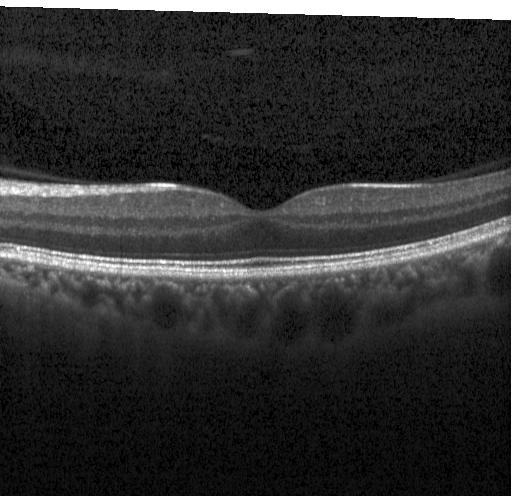

Macular scan. OCT B-scan. Heidelberg Spectralis. SD-OCT
Diagnosis: no choroidal neovascularization, no diabetic macular edema, and no drusen.